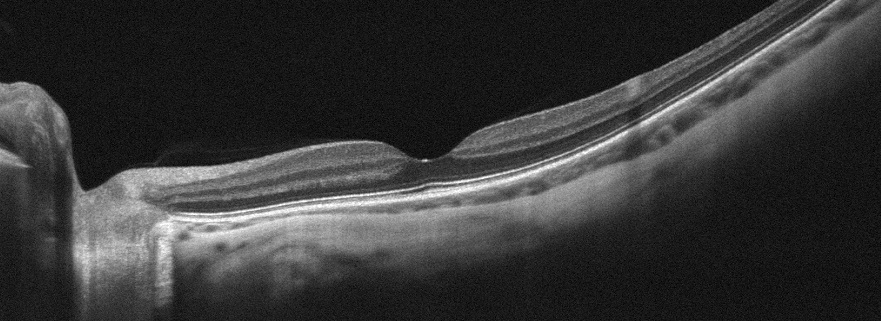
Retinal OCT cross-section; through the macula. This B-scan demonstrates no evidence of AMD, DME, ERM, RAO, RVO, or VID.